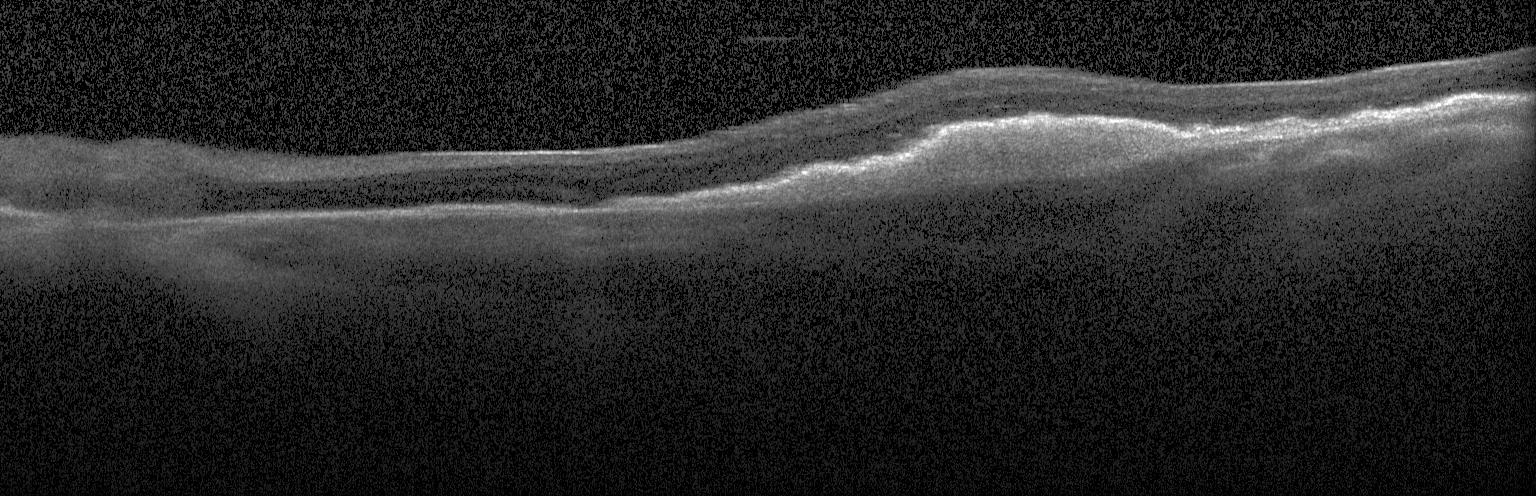 Diagnosis: CNV.